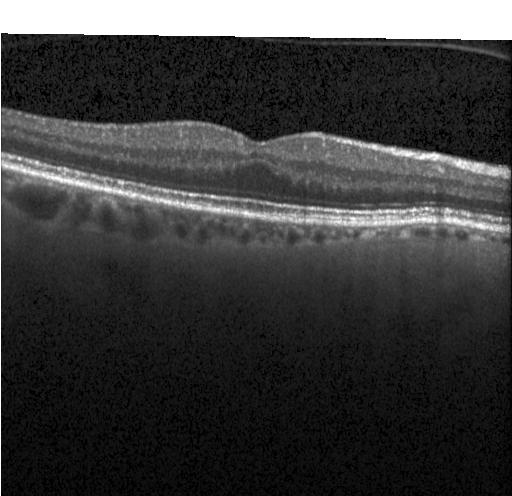

Horizontal scan through the fovea; instrument: Heidelberg Spectralis; spectral-domain optical coherence tomography; optical coherence tomography scan
Neither CNV, DME, nor drusen.